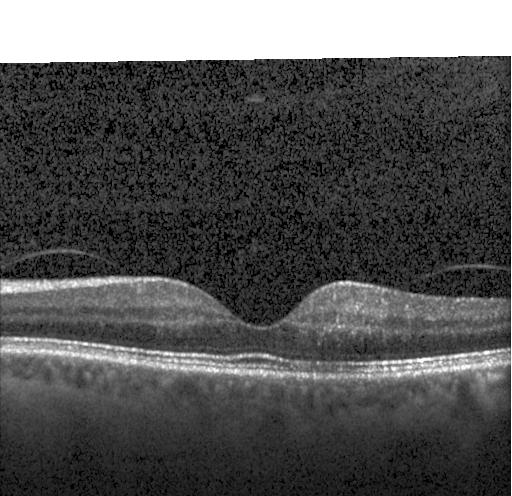
Acquired on a Heidelberg Spectralis · SD-OCT · OCT line scan — This B-scan demonstrates no evidence of choroidal neovascularization, diabetic macular edema, or drusen.